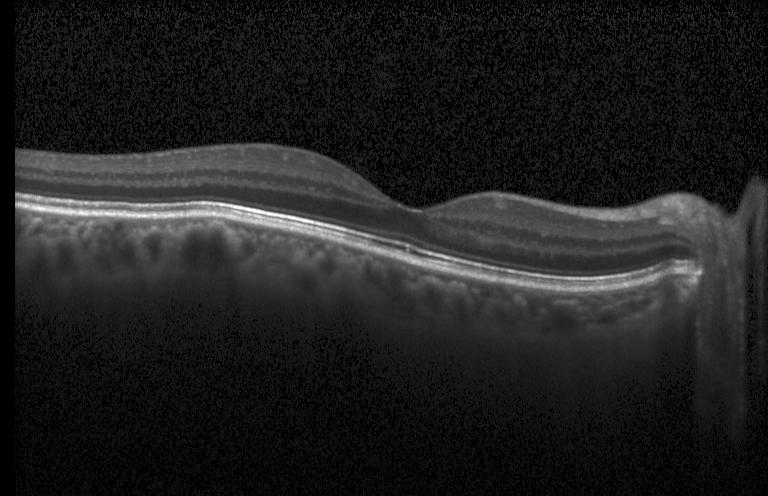

Spectral-domain OCT B-scan: no CNV, DME, or drusen.